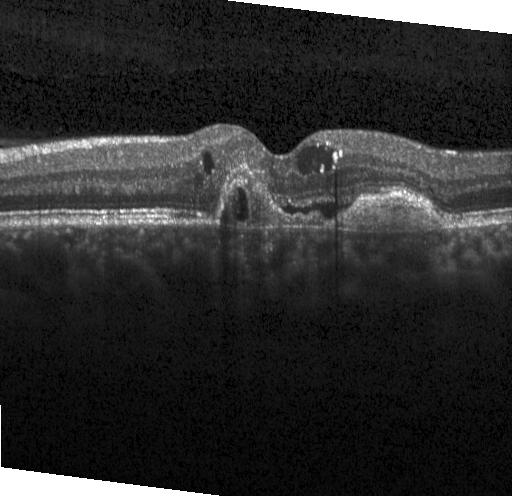
The scan shows choroidal neovascularization (CNV).